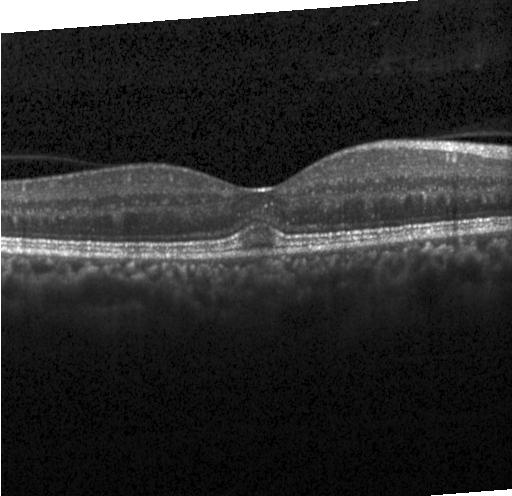

Retinal OCT cross-section; instrument: Heidelberg Spectralis; spectral-domain optical coherence tomography.
The scan shows choroidal neovascularization (CNV).